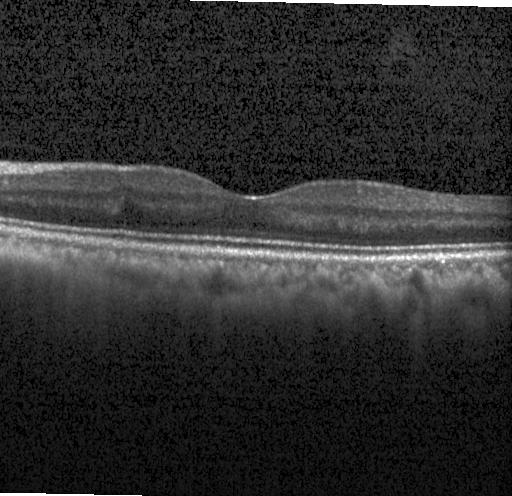
OCT line scan
Dx: no evidence of choroidal neovascularization, diabetic macular edema, or drusen.